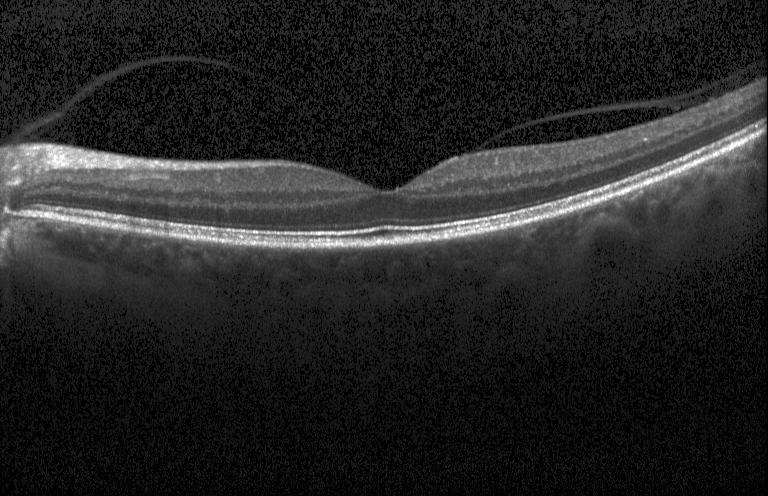
Retinal OCT cross-section; instrument: Heidelberg Spectralis.
Impression: no CNV, DME, or drusen.